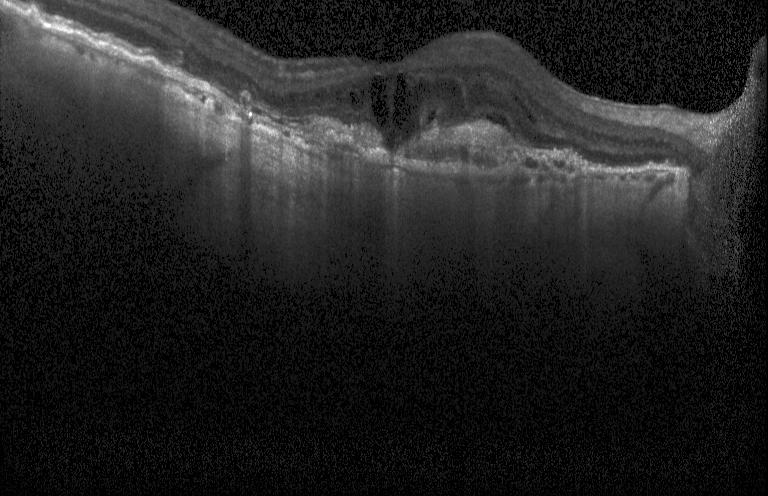 Retinal OCT B-scan
Impression: choroidal neovascularization.